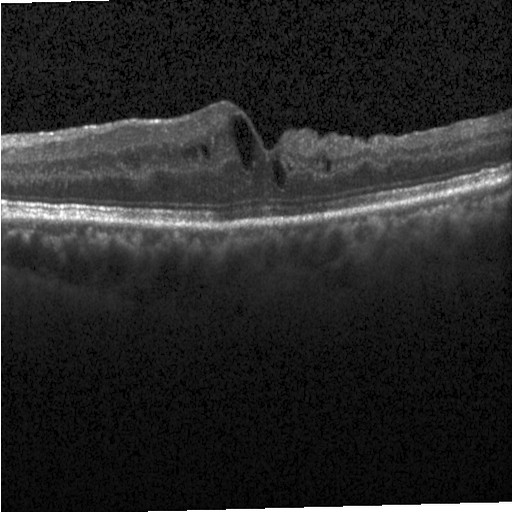
Impression: diabetic macular edema.